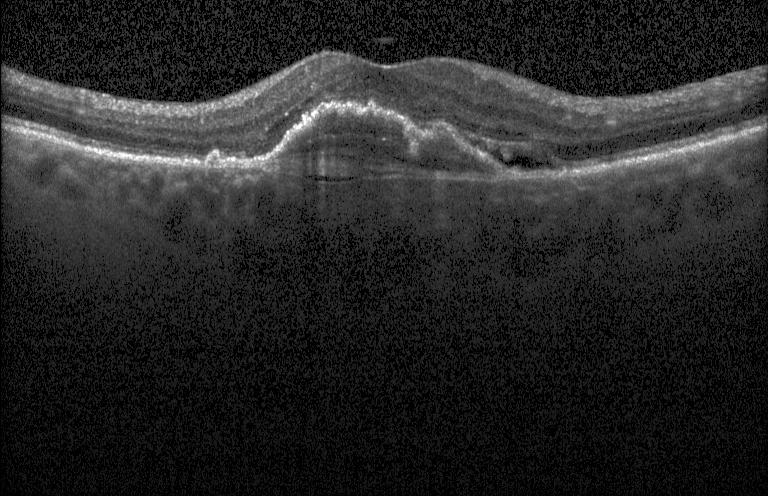
Retinal OCT cross-section.
The scan shows choroidal neovascularization.